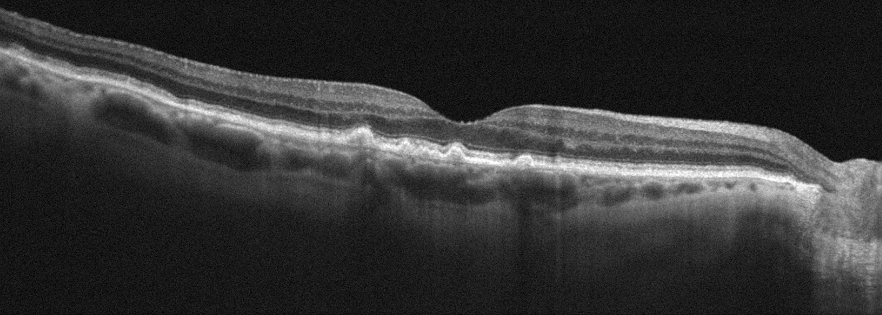 Finding: age-related macular degeneration.